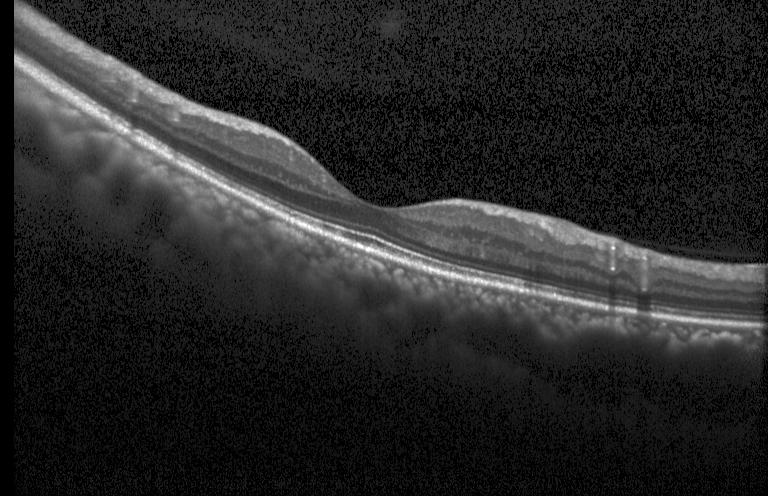
Optical coherence tomography B-scan. Impression: neither choroidal neovascularization, diabetic macular edema, nor drusen.